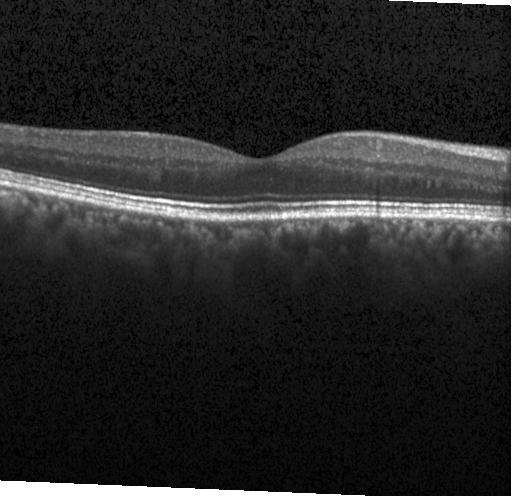
Finding: neither choroidal neovascularization, diabetic macular edema, nor drusen.